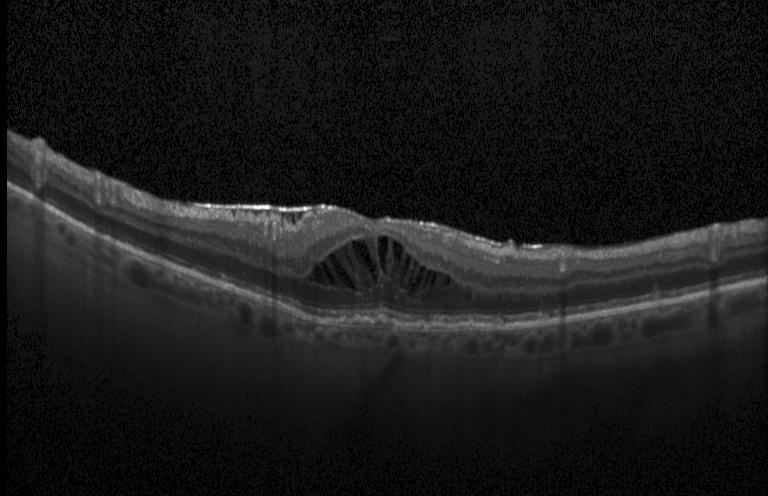

Through the macula · retinal OCT cross-section — Diagnosis: DME.